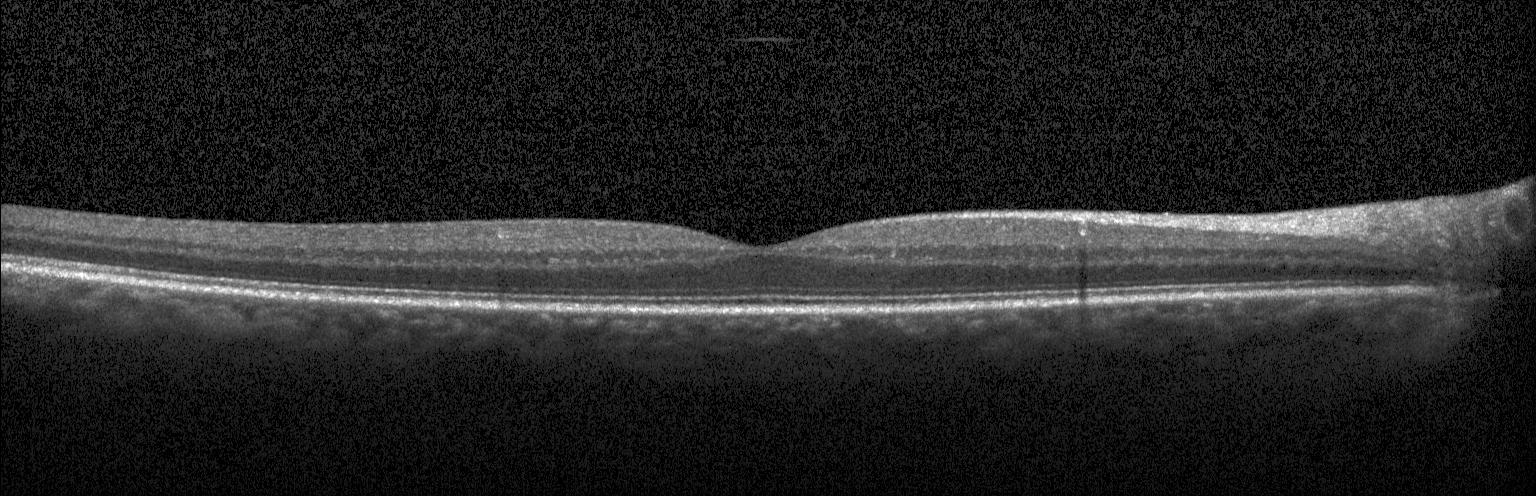

Macular OCT demonstrating no choroidal neovascularization, diabetic macular edema, or drusen.